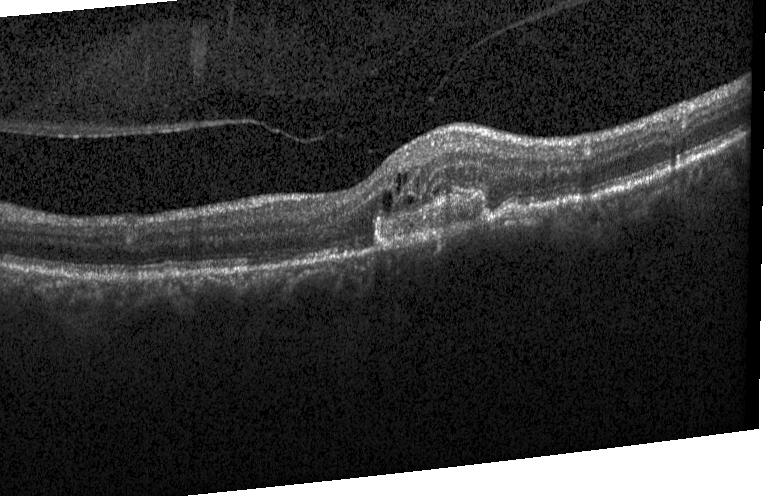
OCT line scan, centered on the fovea, SD-OCT. Finding: a choroidal neovascular membrane.